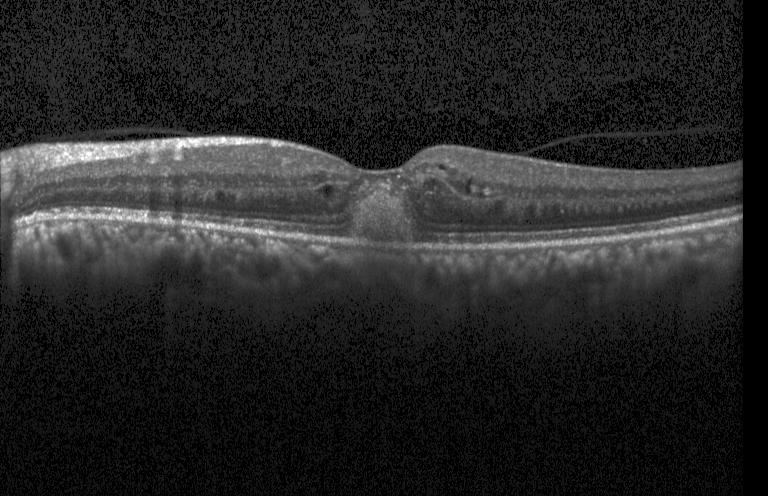

Optical coherence tomography B-scan.
OCT finding: CNV.